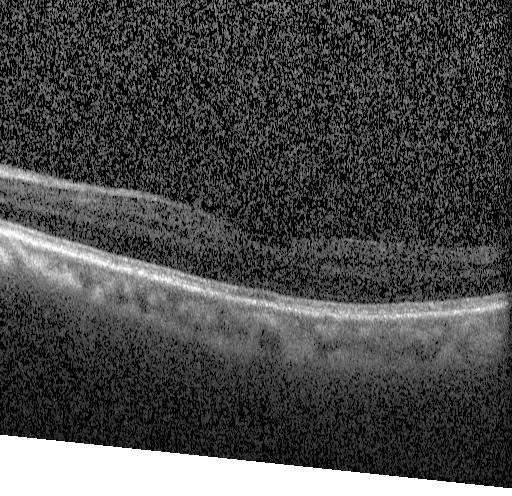
Optical coherence tomography B-scan
Dx: neither choroidal neovascularization, diabetic macular edema, nor drusen.